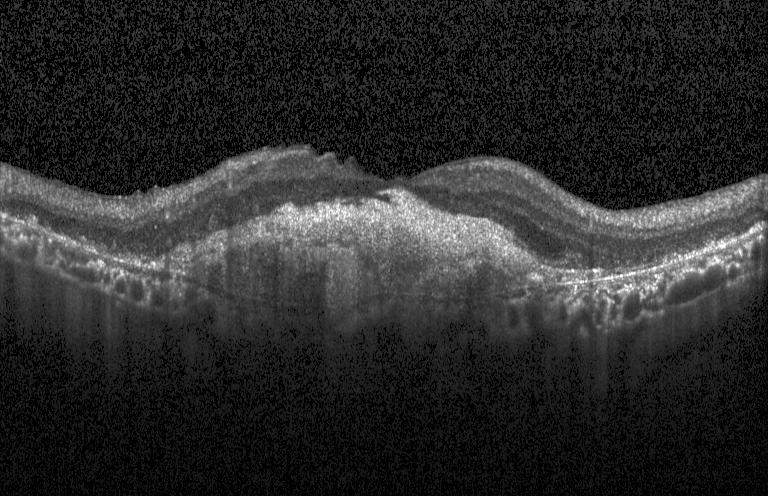 Macular scan, OCT line scan.
Finding: choroidal neovascularization (CNV).